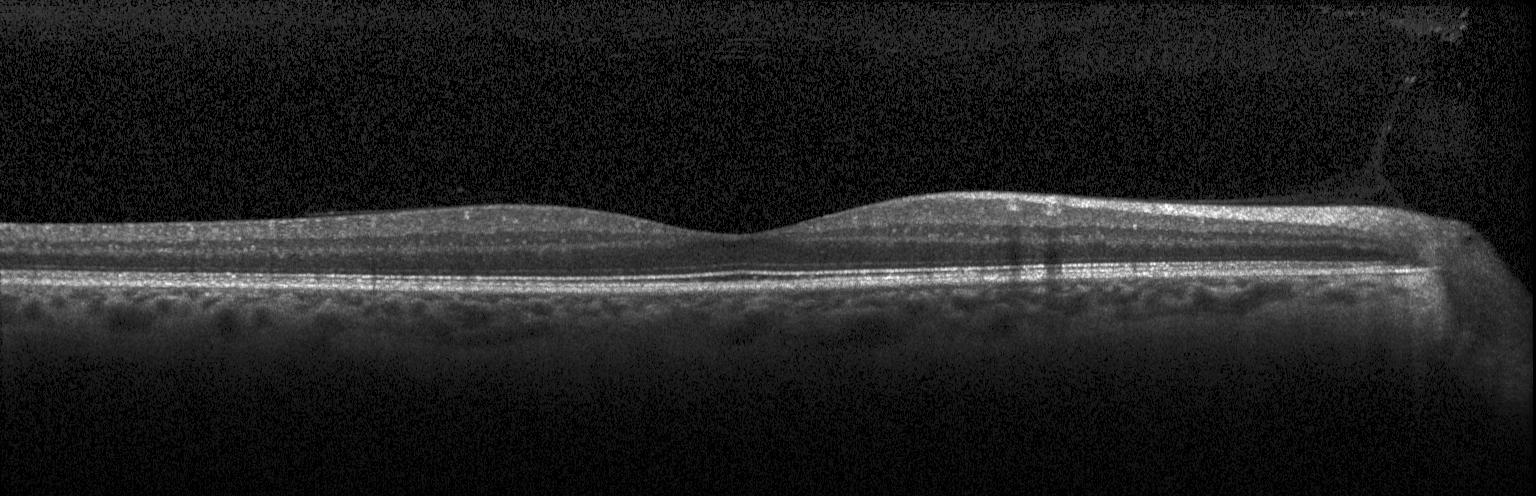 This B-scan demonstrates no choroidal neovascularization, diabetic macular edema, or drusen.